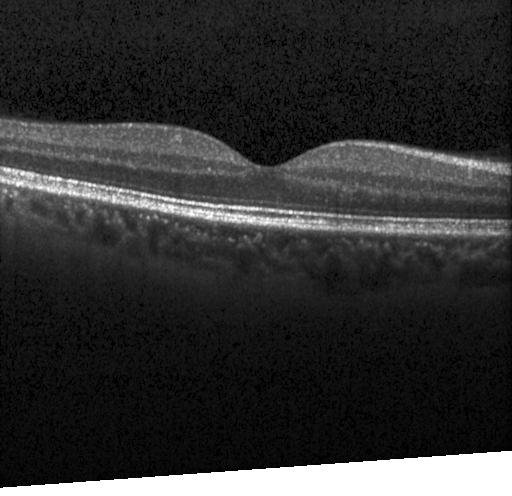 Retinal OCT cross-section showing no choroidal neovascularization, diabetic macular edema, or drusen.